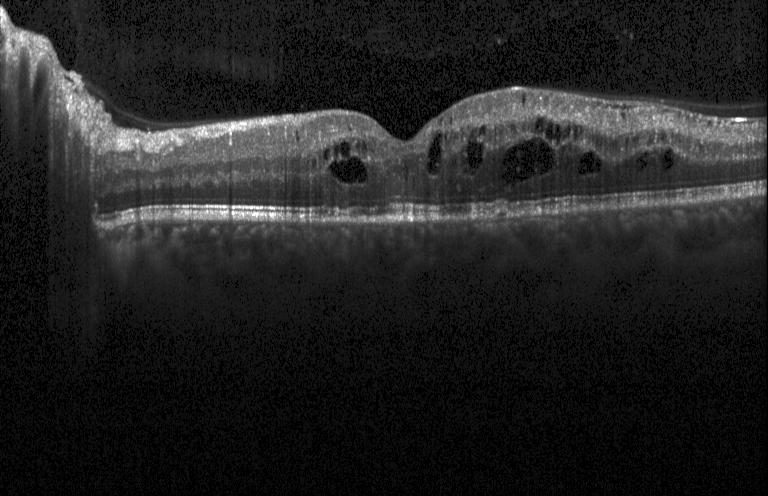

OCT B-scan. Macular scan. Instrument: Heidelberg Spectralis. Spectral-domain OCT.
Finding: DME.